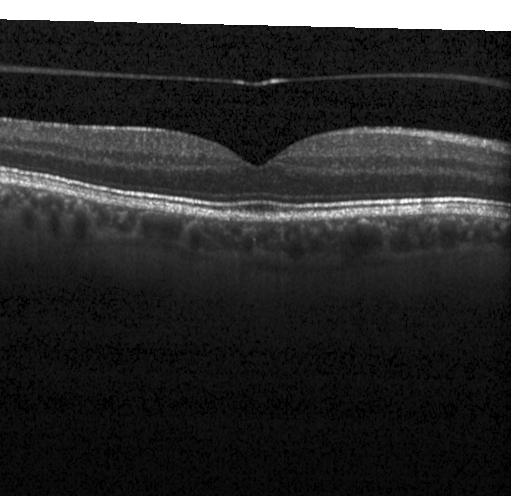

OCT line scan. Finding: no evidence of CNV, DME, or drusen.